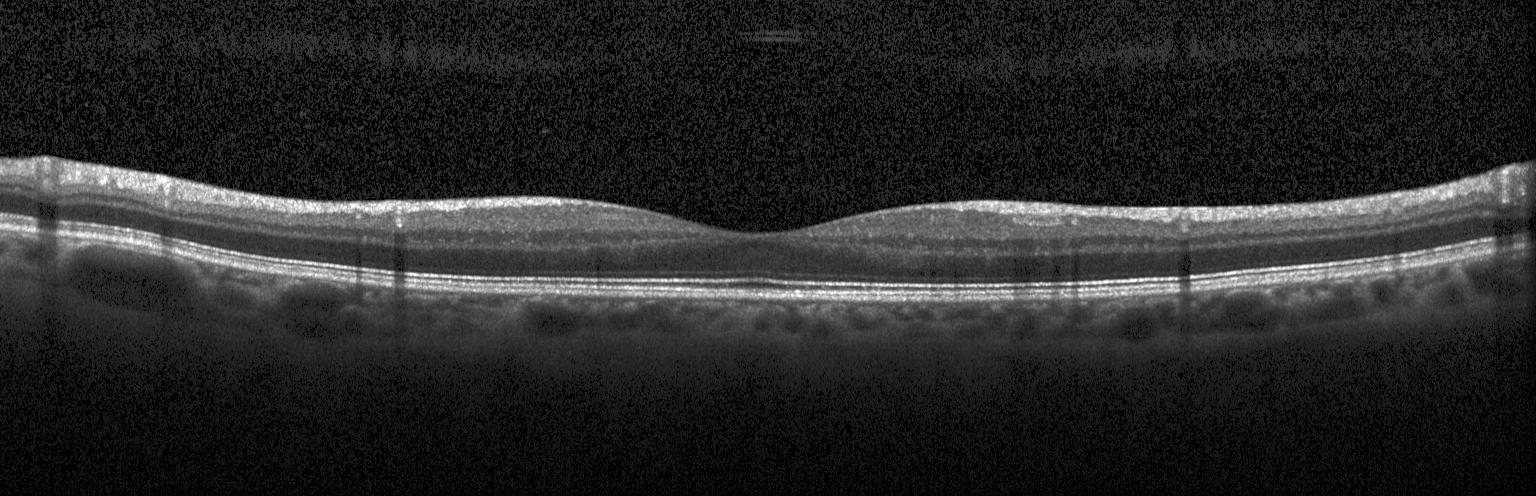

Acquired on a Heidelberg Spectralis, optical coherence tomography B-scan, fovea-centered, spectral-domain optical coherence tomography — Macular OCT: no CNV, no DME, and no drusen.